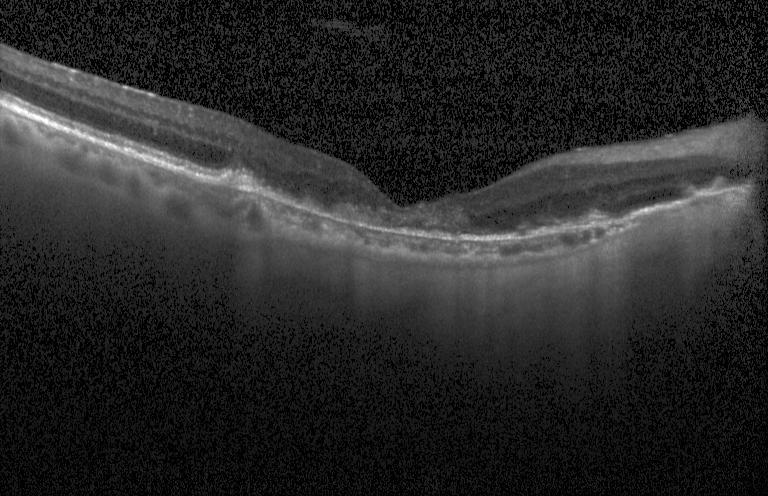

Retinal OCT cross-section; macular scan; SD-OCT; instrument: Heidelberg Spectralis.
OCT finding: choroidal neovascularization (CNV).